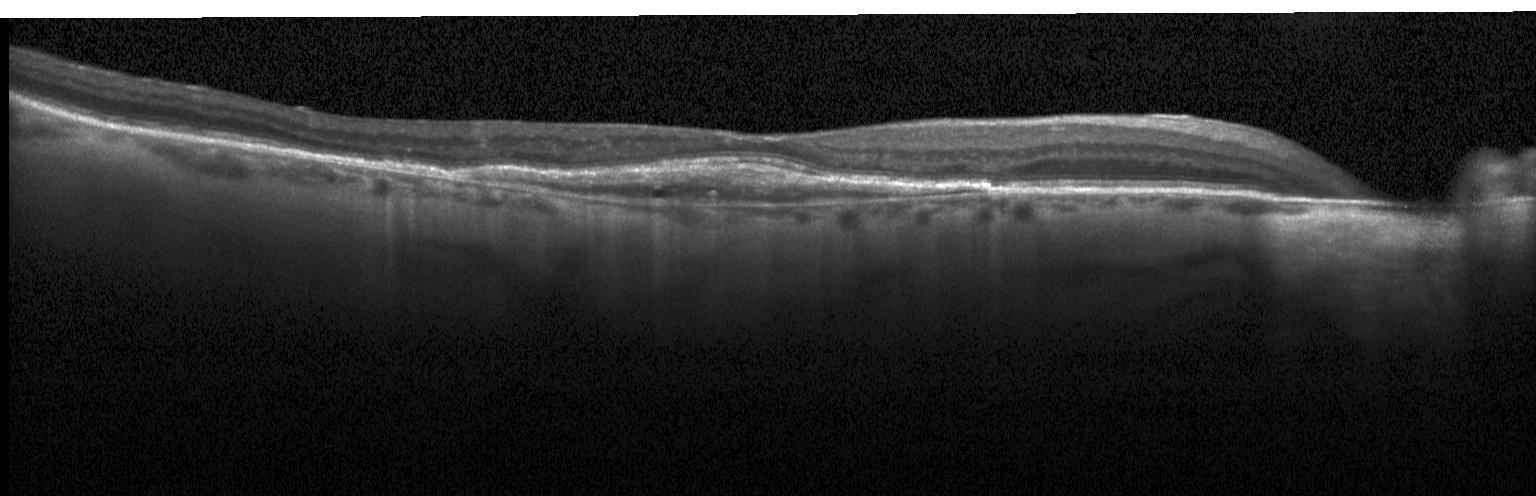
OCT B-scan
Choroidal neovascularization (CNV).